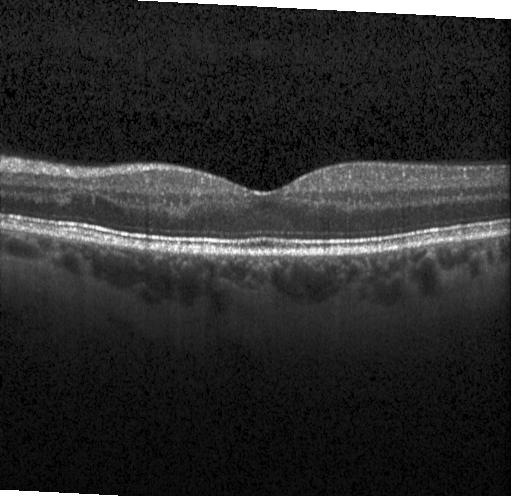

Acquired on a Heidelberg Spectralis · optical coherence tomography B-scan · spectral-domain optical coherence tomography
Impression: no choroidal neovascularization, diabetic macular edema, or drusen.